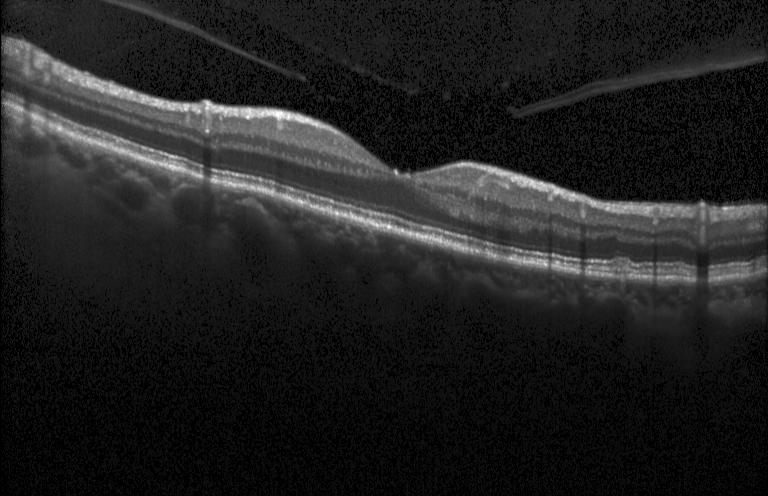
Fovea-centered; OCT line scan; spectral-domain optical coherence tomography — Impression: sub-RPE drusenoid deposits.